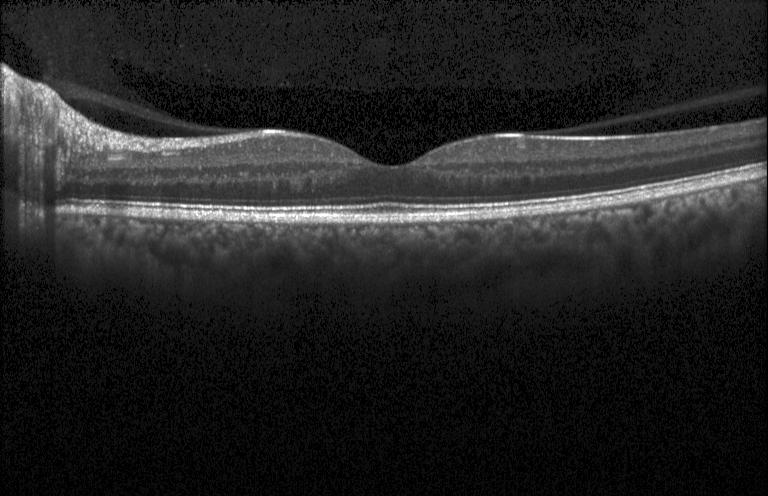
Optical coherence tomography scan. This B-scan demonstrates neither choroidal neovascularization, diabetic macular edema, nor drusen.